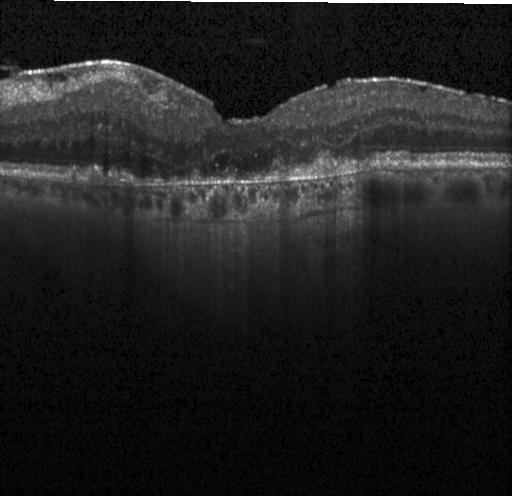 This B-scan demonstrates choroidal neovascularization (CNV).